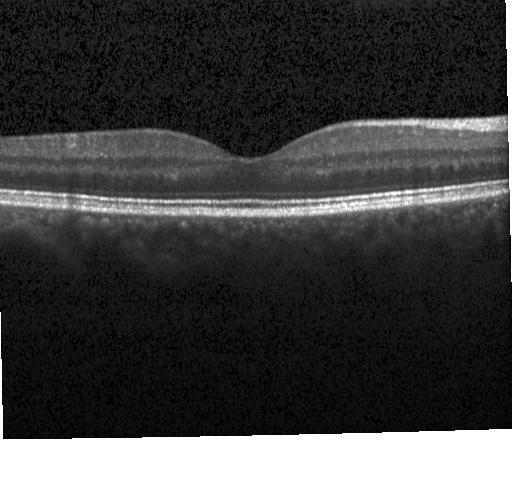

Instrument: Heidelberg Spectralis · retinal OCT cross-section · spectral-domain OCT
Dx: no CNV, DME, or drusen.